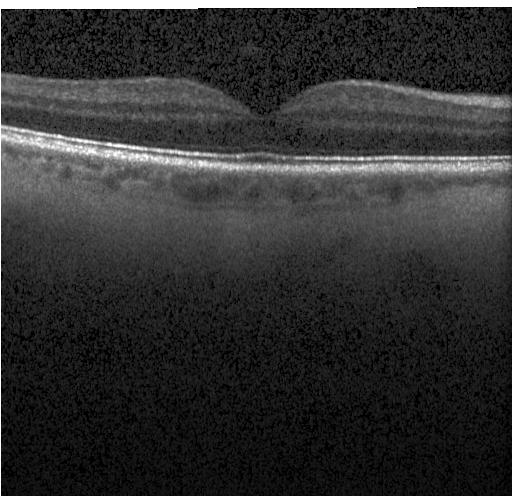 Optical coherence tomography B-scan. Assessment: no evidence of choroidal neovascularization, diabetic macular edema, or drusen.